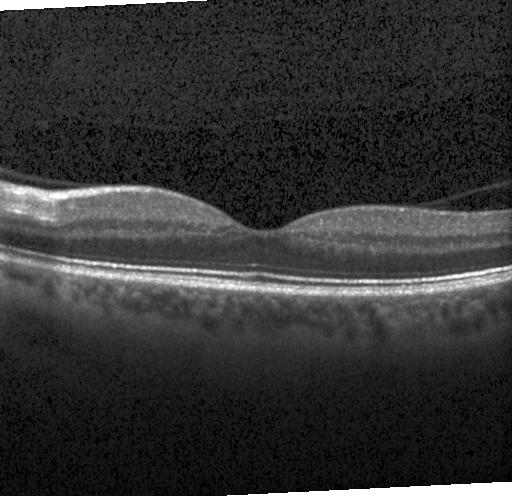

Spectral-domain optical coherence tomography; retinal OCT cross-section; macular scan.
Assessment: no evidence of choroidal neovascularization, diabetic macular edema, or drusen.